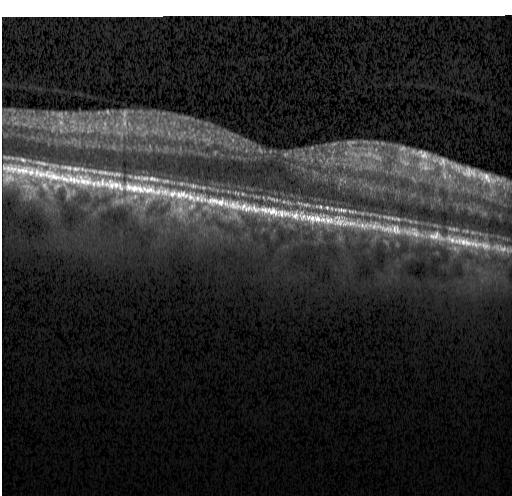 SD-OCT · optical coherence tomography B-scan.
No evidence of choroidal neovascularization, diabetic macular edema, or drusen.